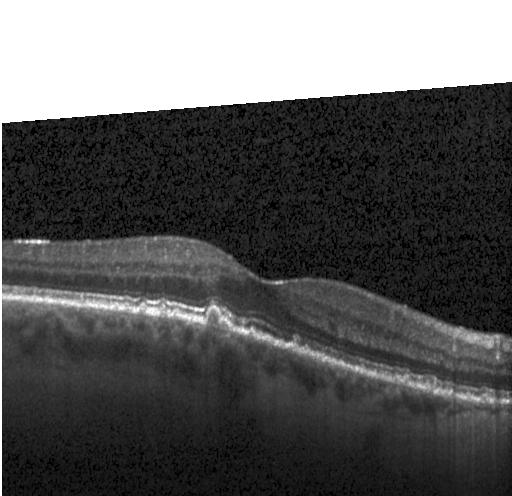
Optical coherence tomography scan. Acquired on a Heidelberg Spectralis.
Diagnosis: sub-RPE drusenoid deposits.